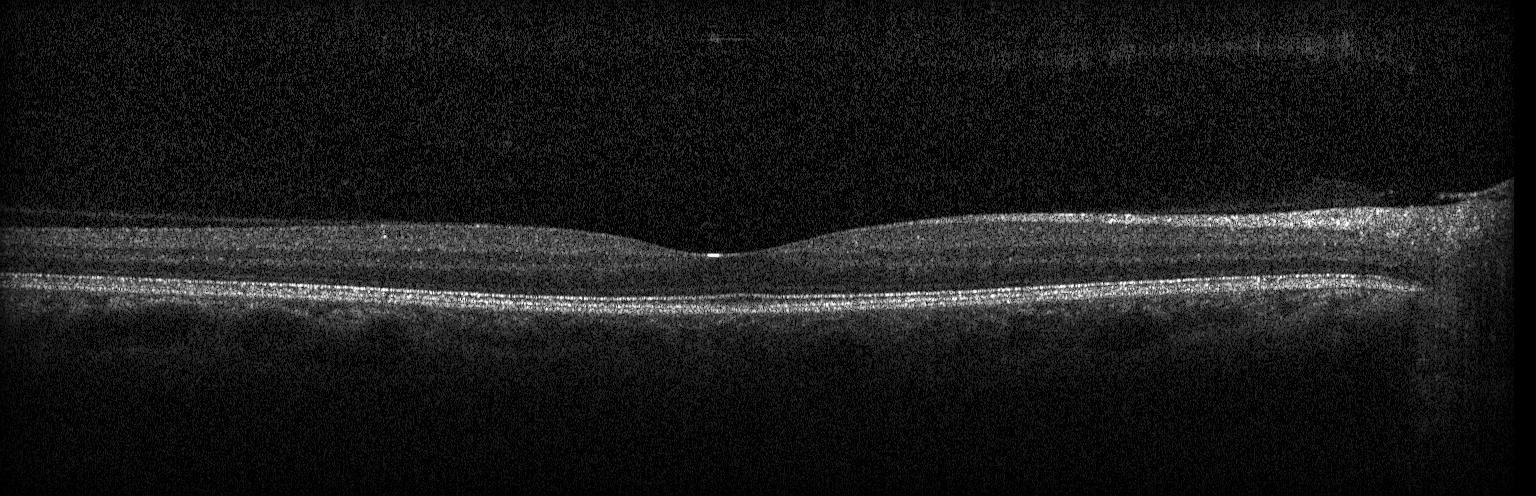

Spectral-domain optical coherence tomography, retinal OCT cross-section — Diagnosis: no choroidal neovascularization, no diabetic macular edema, and no drusen.